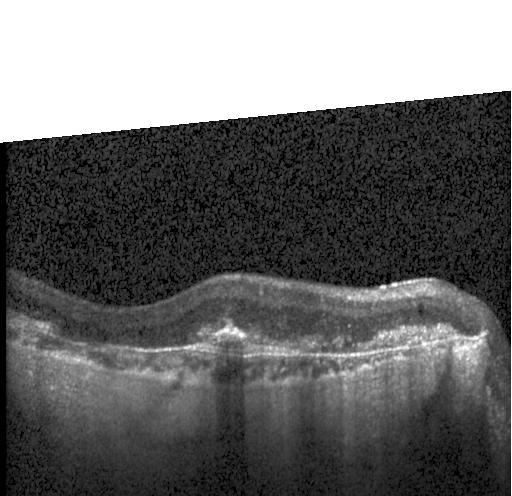
SD-OCT · instrument: Heidelberg Spectralis · retinal OCT B-scan. The scan shows a choroidal neovascular membrane.